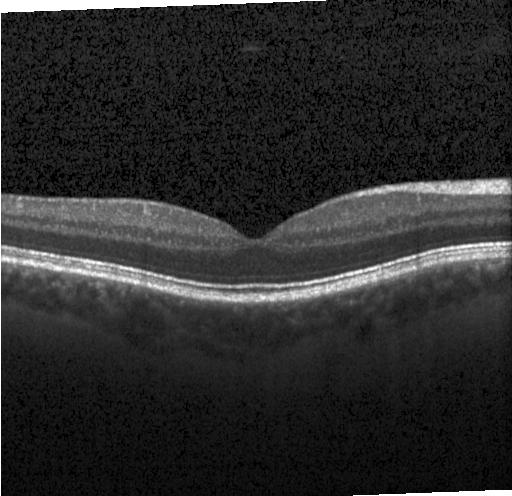
No evidence of CNV, DME, or drusen.